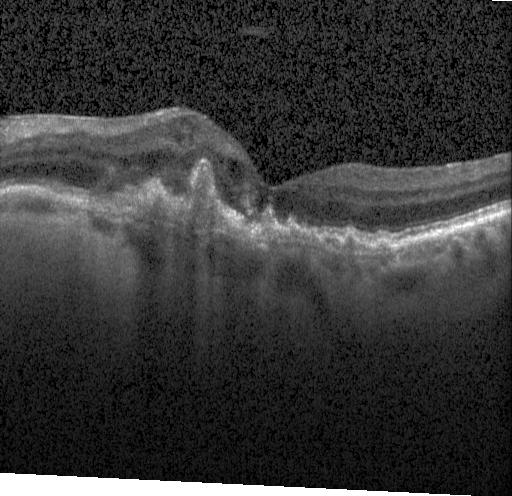
This B-scan demonstrates a choroidal neovascular membrane.